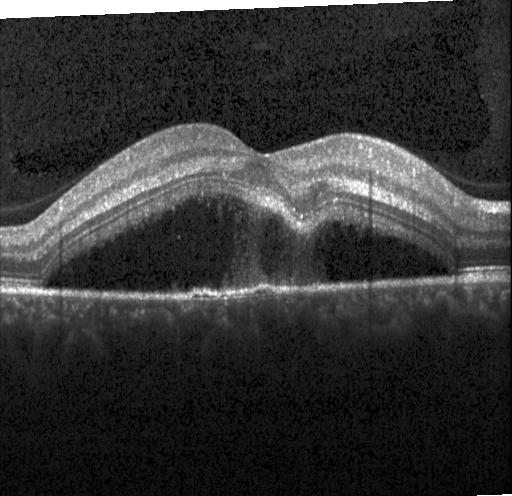 Macular OCT demonstrating a choroidal neovascular membrane.